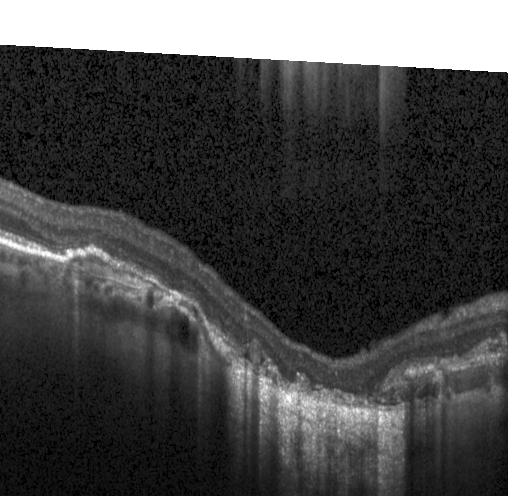 Optical coherence tomography B-scan. Dx: a choroidal neovascular membrane.